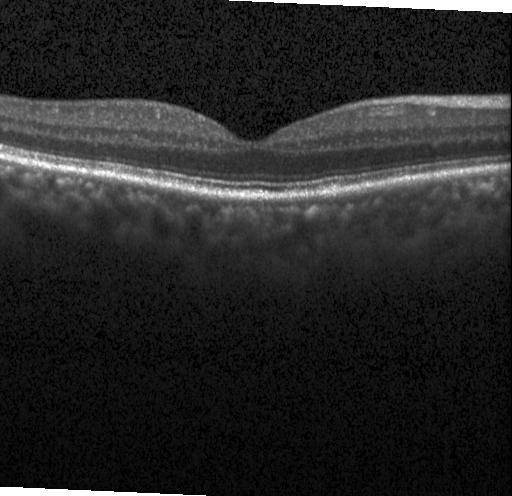 Retinal OCT B-scan. Spectral-domain OCT. Heidelberg Spectralis.
Diagnosis: no choroidal neovascularization, no diabetic macular edema, and no drusen.